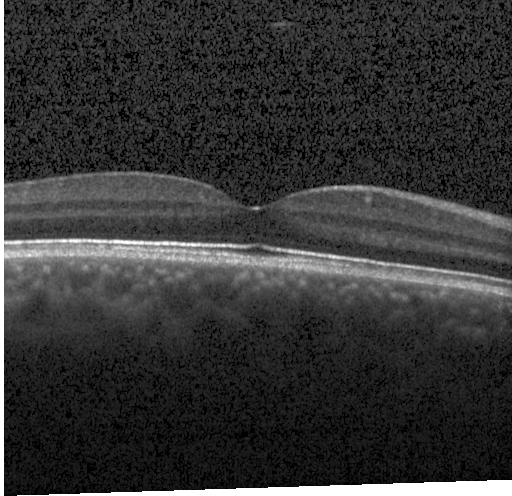

Optical coherence tomography B-scan; SD-OCT
Impression: neither CNV, DME, nor drusen.